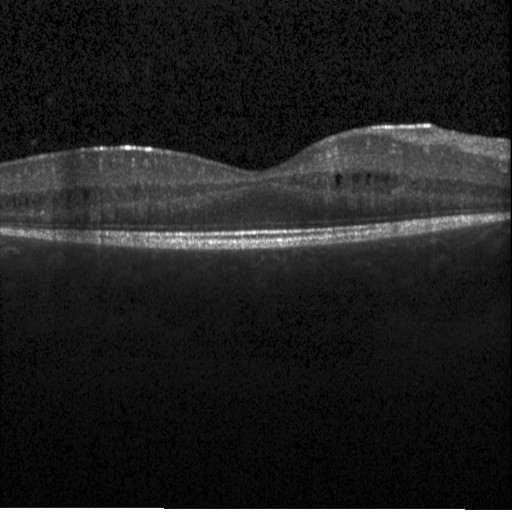

Retinal OCT B-scan, acquired on a Heidelberg Spectralis. Impression: diabetic macular edema.